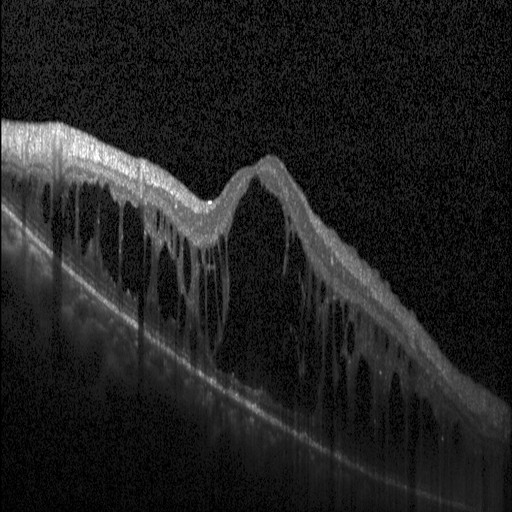 Spectral-domain OCT; acquired on a Heidelberg Spectralis; retinal OCT cross-section. DME.